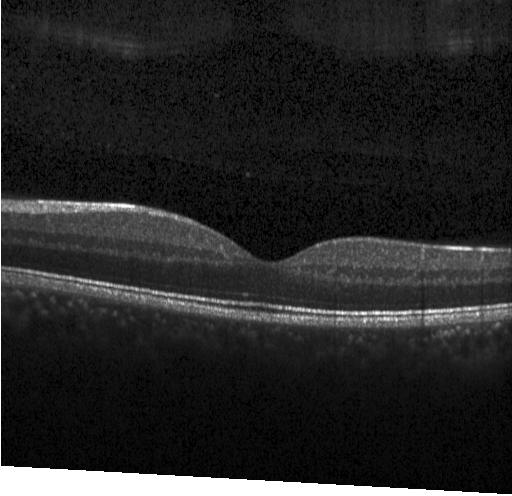
Acquired on a Heidelberg Spectralis, spectral-domain OCT, macular scan, optical coherence tomography scan
This B-scan demonstrates no CNV, no DME, and no drusen.